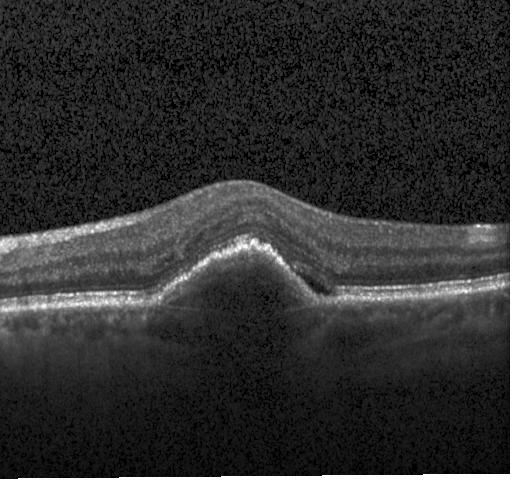 Retinal OCT B-scan.
Diagnosis: choroidal neovascularization.